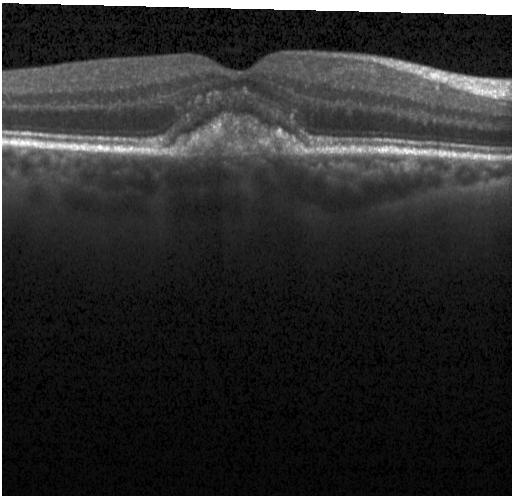
Spectral-domain OCT. Heidelberg Spectralis. Optical coherence tomography scan. Fovea-centered — Diagnosis: CNV.